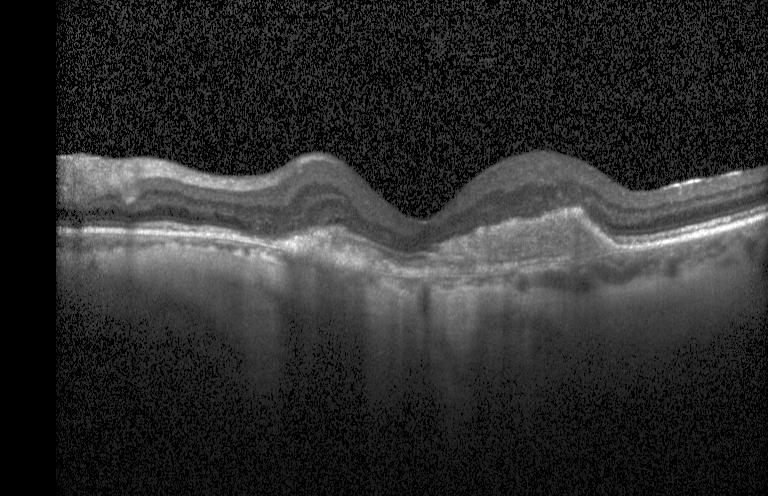

Through the macula · OCT B-scan · Heidelberg Spectralis.
Diagnosis: a choroidal neovascular membrane.